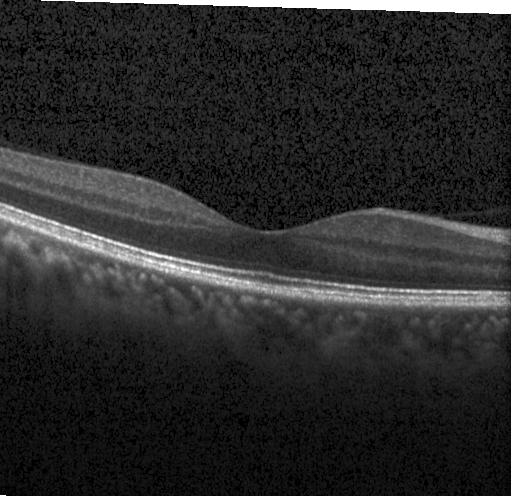
OCT finding: no evidence of choroidal neovascularization, diabetic macular edema, or drusen.